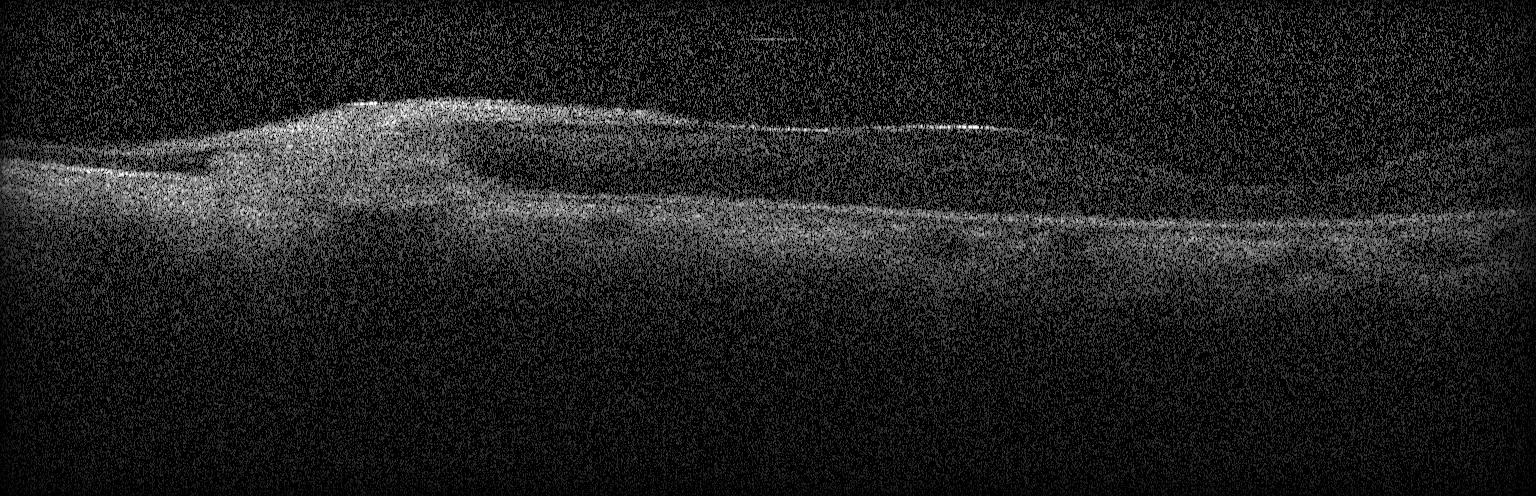 Optical coherence tomography B-scan
Diagnosis: a choroidal neovascular membrane.